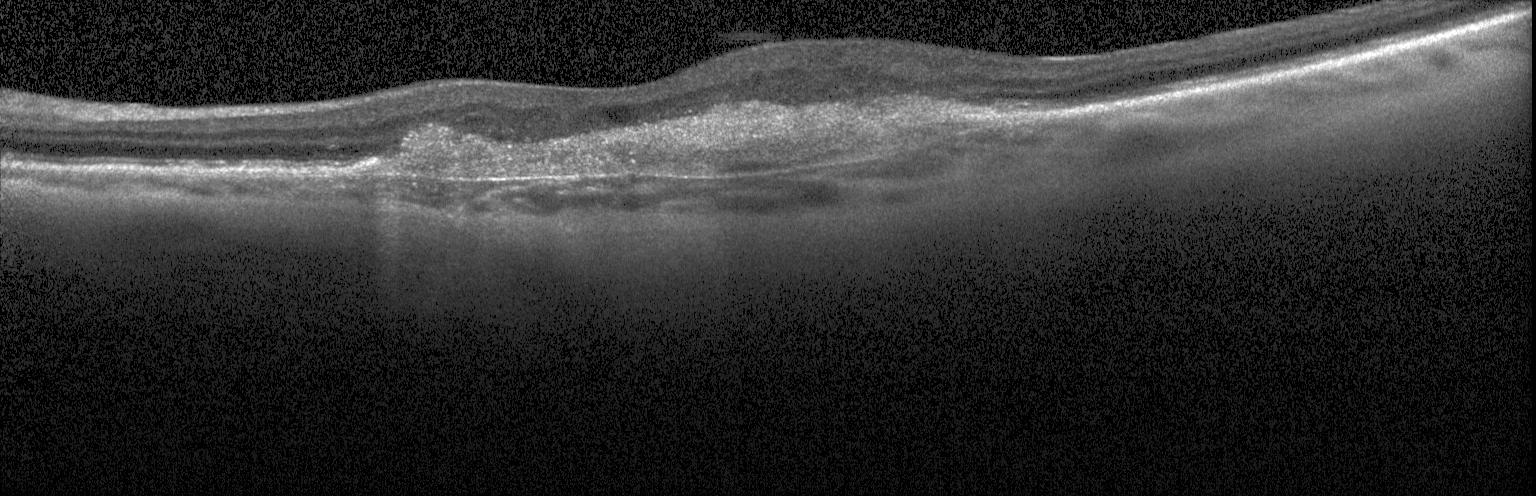

Macular scan. Retinal OCT B-scan. Heidelberg Spectralis OCT system
Assessment: a choroidal neovascular membrane.